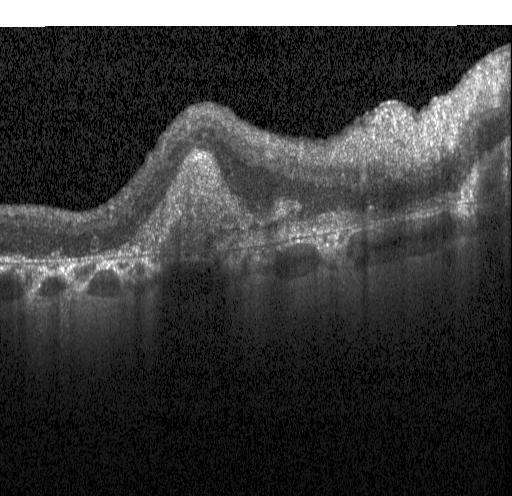

Optical coherence tomography scan — The scan shows choroidal neovascularization (CNV).